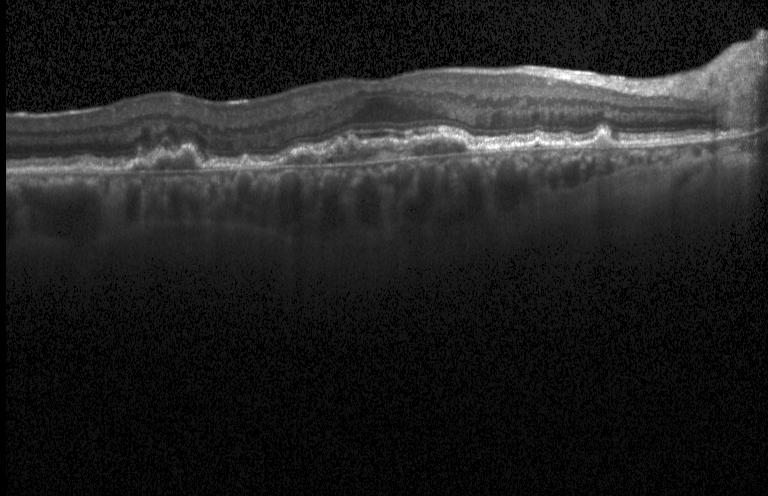

OCT scan showing a choroidal neovascular membrane.